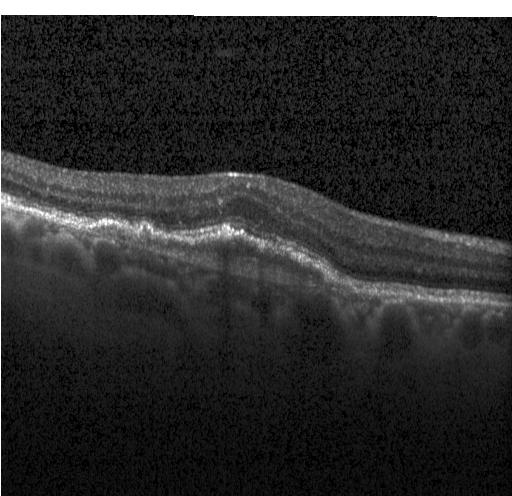
Spectral-domain OCT B-scan: choroidal neovascularization.